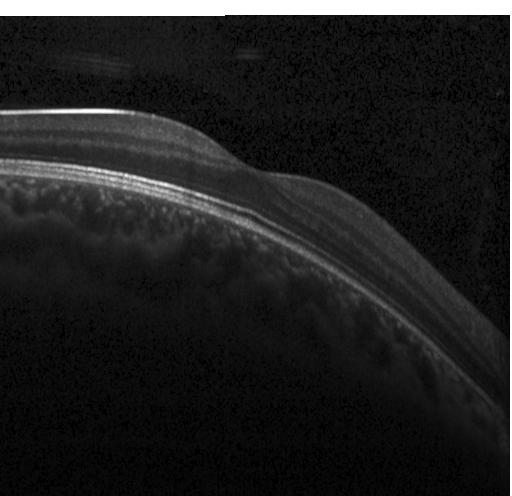
Fovea-centered. Retinal OCT B-scan.
Diagnosis: neither CNV, DME, nor drusen.